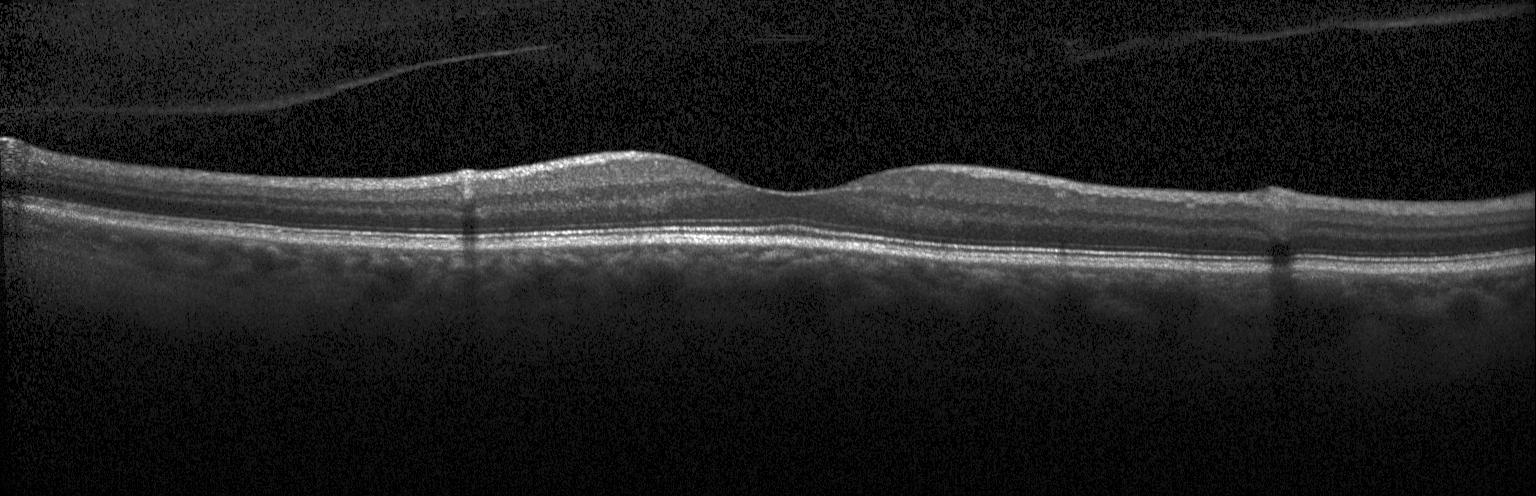

Dx: neither choroidal neovascularization, diabetic macular edema, nor drusen.